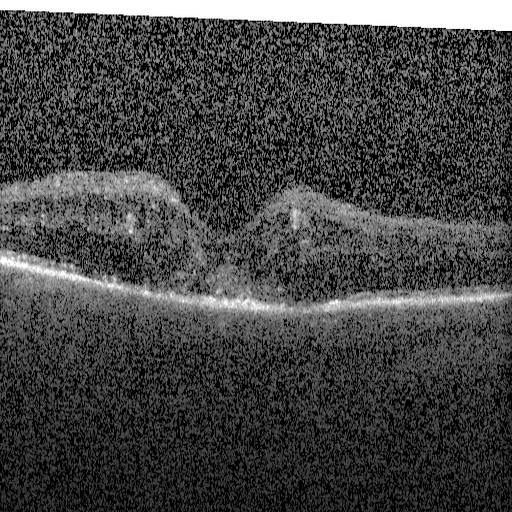

Acquired on a Heidelberg Spectralis · retinal OCT cross-section · horizontal scan through the fovea
Impression: diabetic macular edema (DME).